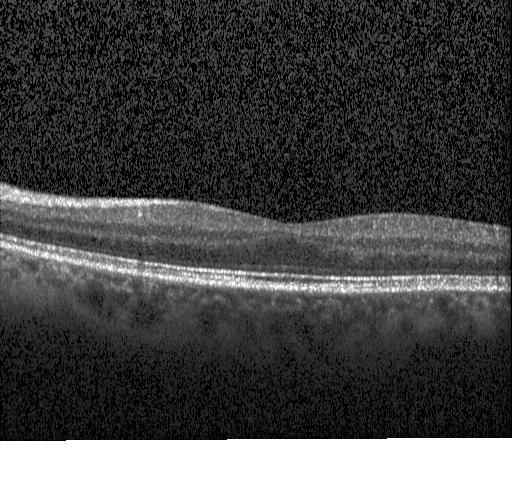
Finding: no choroidal neovascularization, no diabetic macular edema, and no drusen.